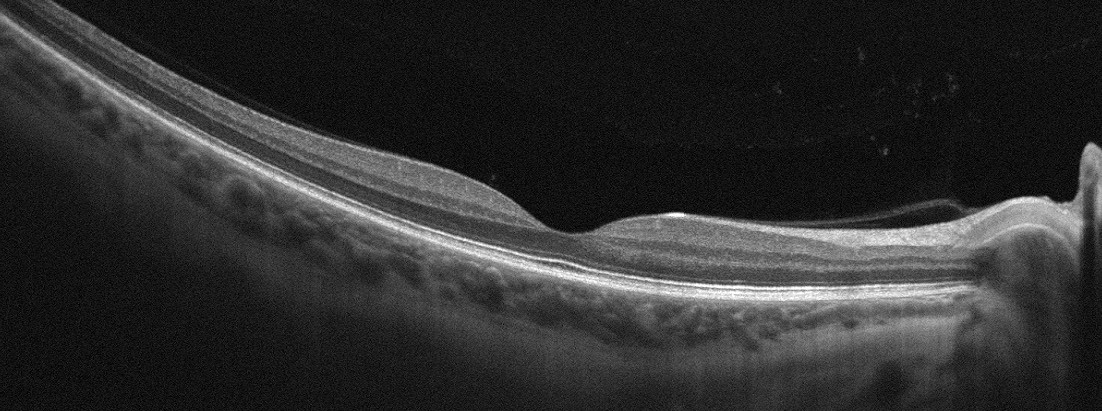
Optical coherence tomography B-scan. Macular scan. Macular OCT: no evidence of AMD, DME, ERM, RAO, RVO, or VID.